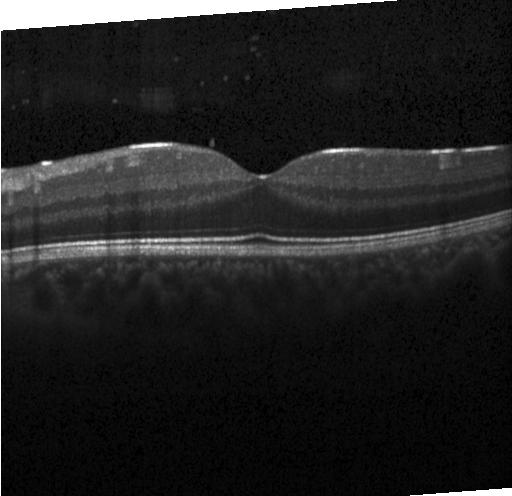

OCT B-scan showing no evidence of choroidal neovascularization, diabetic macular edema, or drusen.